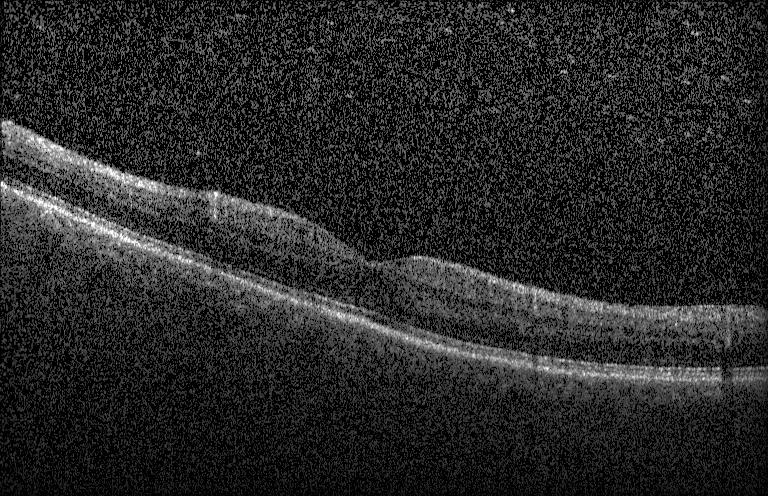
SD-OCT, acquired on a Heidelberg Spectralis, centered on the fovea, OCT B-scan
Dx: neither choroidal neovascularization, diabetic macular edema, nor drusen.